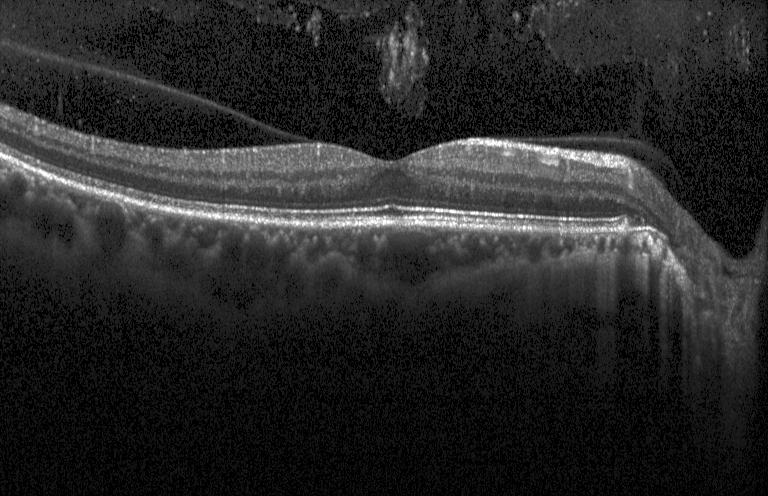

Diagnosis: no evidence of choroidal neovascularization, diabetic macular edema, or drusen.